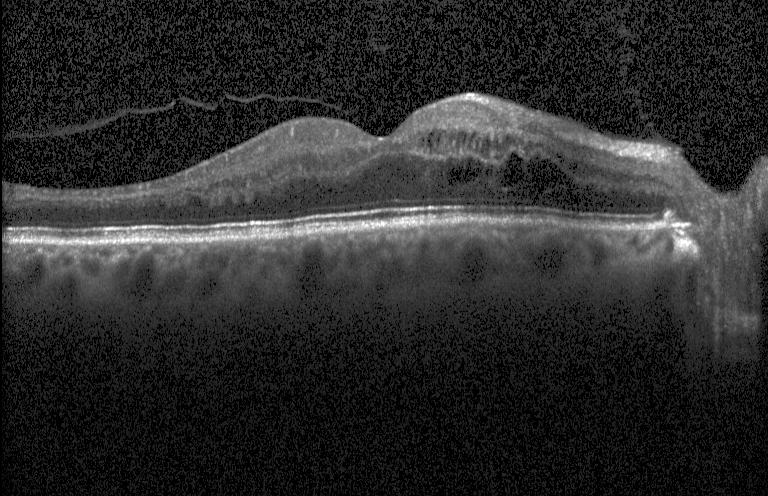 Dx: DME.